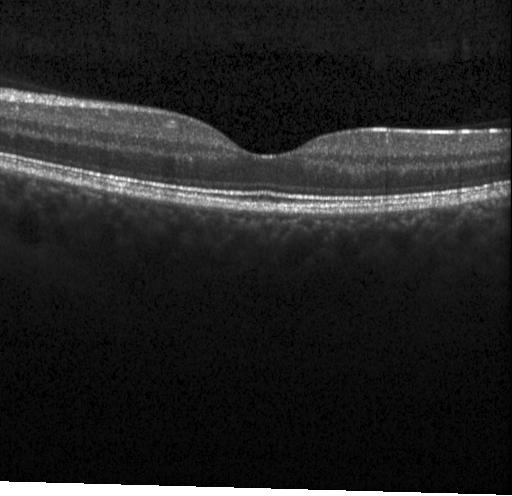

Retinal OCT B-scan.
Finding: no choroidal neovascularization, diabetic macular edema, or drusen.